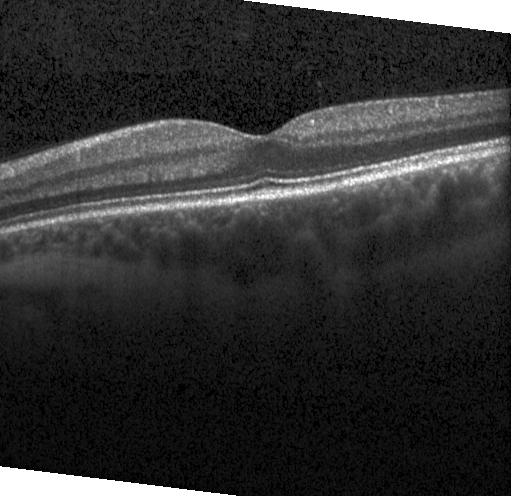
Impression: no evidence of choroidal neovascularization, diabetic macular edema, or drusen.